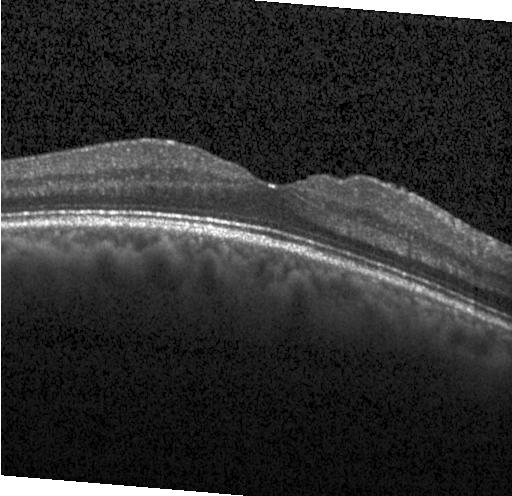 Impression: no choroidal neovascularization, no diabetic macular edema, and no drusen.